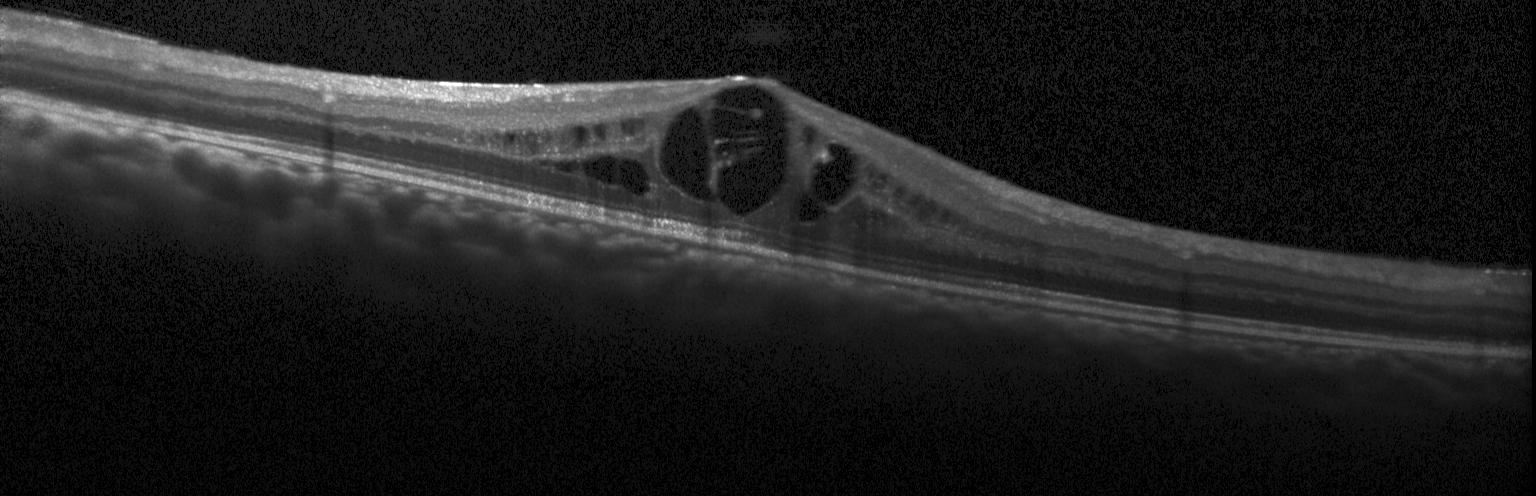

Dx: DME.